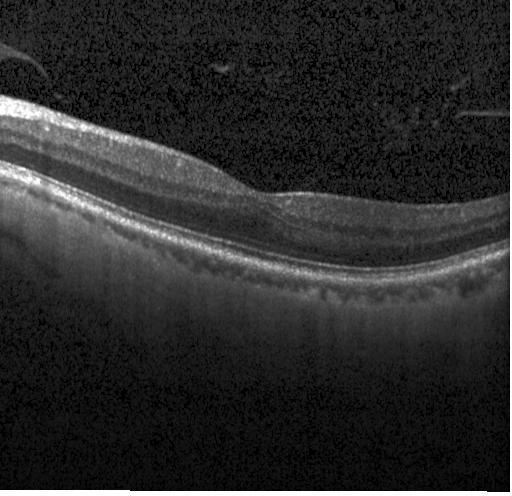

Macular scan · SD-OCT · optical coherence tomography scan · Heidelberg Spectralis
Diagnosis: neither choroidal neovascularization, diabetic macular edema, nor drusen.